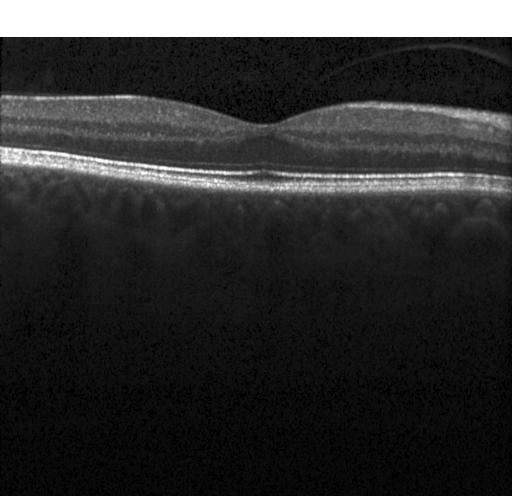 Heidelberg Spectralis, OCT line scan, spectral-domain OCT, fovea-centered.
No choroidal neovascularization, no diabetic macular edema, and no drusen.